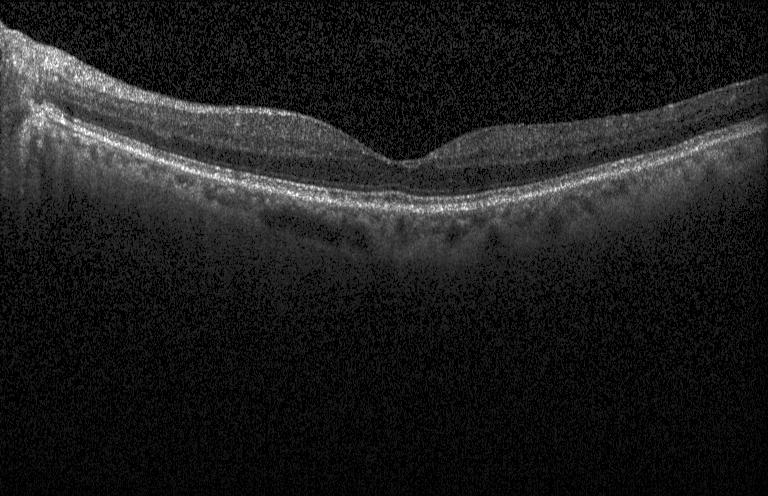

Diagnosis: no evidence of CNV, DME, or drusen.